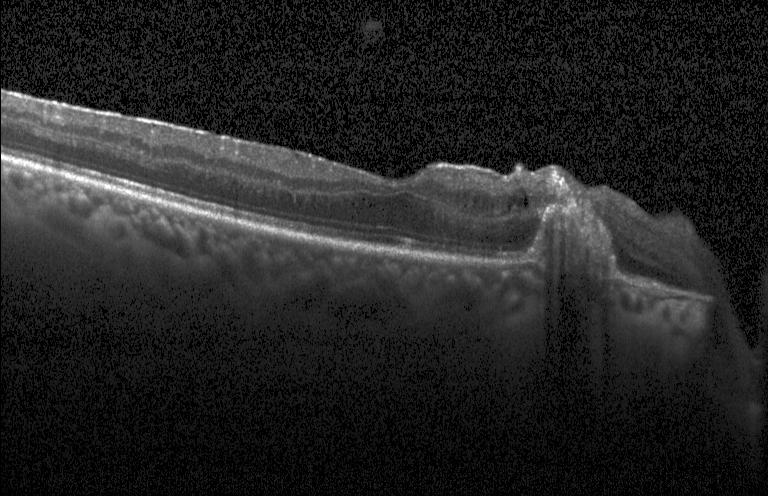
Horizontal scan through the fovea. OCT line scan. Spectral-domain OCT. Heidelberg Spectralis OCT system — Macular OCT: CNV.